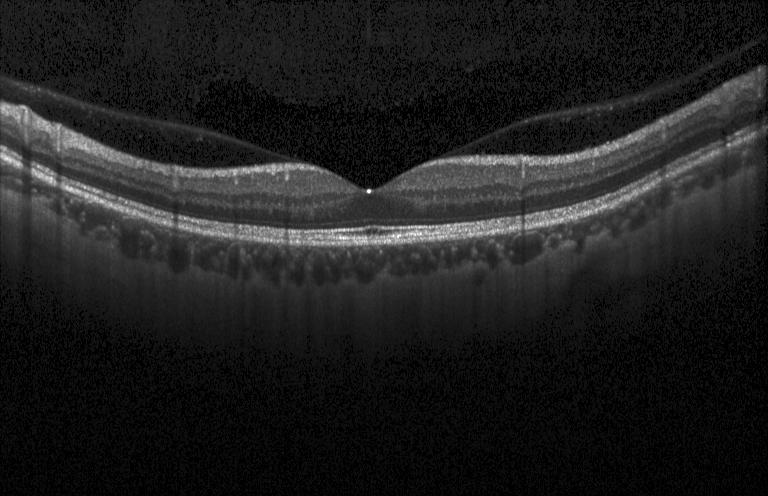 This B-scan demonstrates no choroidal neovascularization, diabetic macular edema, or drusen.